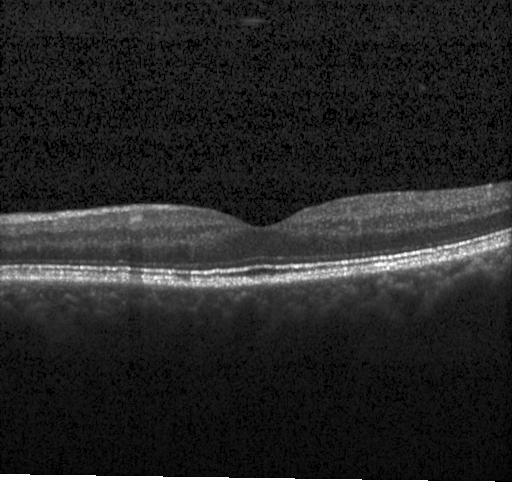
OCT line scan; spectral-domain OCT; fovea-centered.
The scan shows no choroidal neovascularization, diabetic macular edema, or drusen.